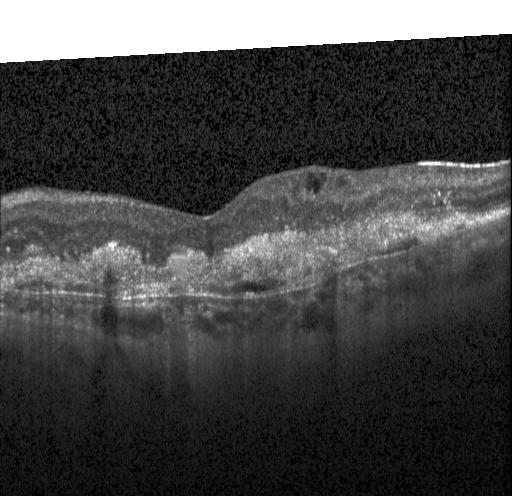 Spectral-domain OCT. Optical coherence tomography scan
Finding: choroidal neovascularization.